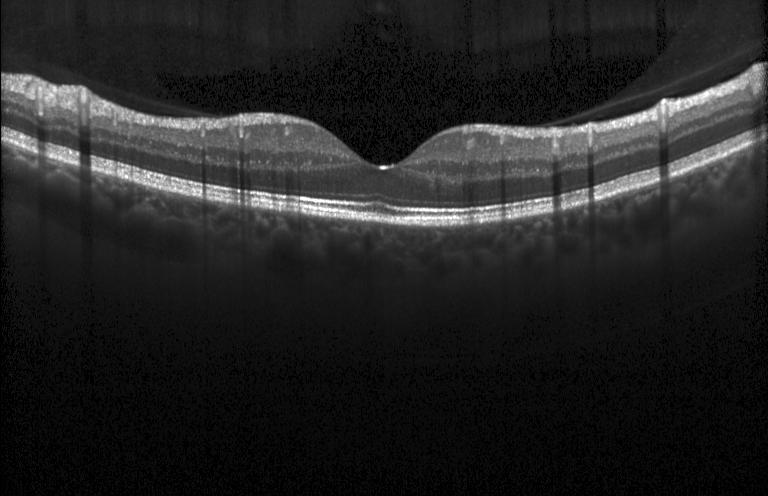

Spectral-domain OCT · centered on the fovea · optical coherence tomography scan.
Finding: no evidence of choroidal neovascularization, diabetic macular edema, or drusen.